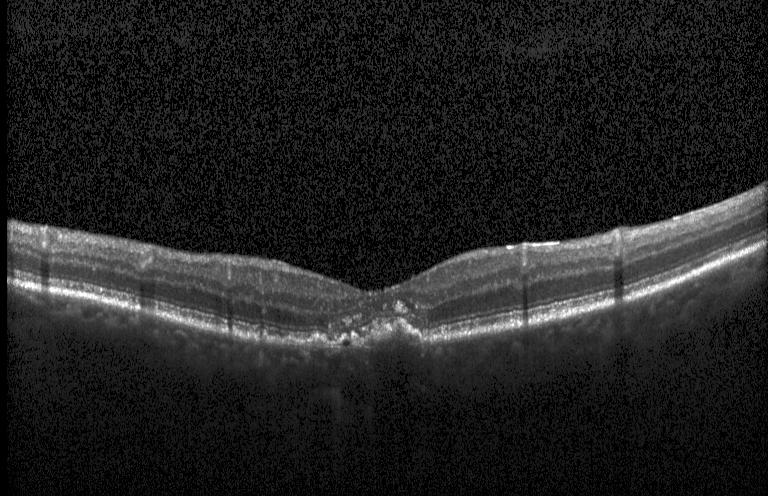 Fovea-centered · spectral-domain OCT · OCT B-scan.
Macular OCT: a choroidal neovascular membrane.